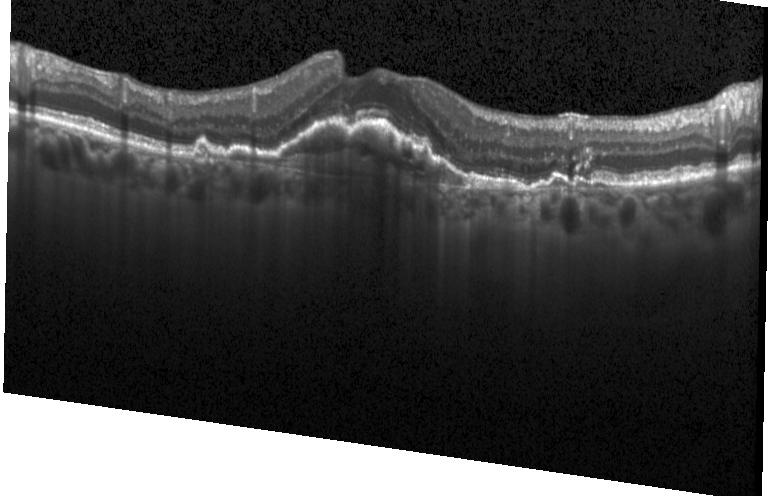

OCT finding: CNV.